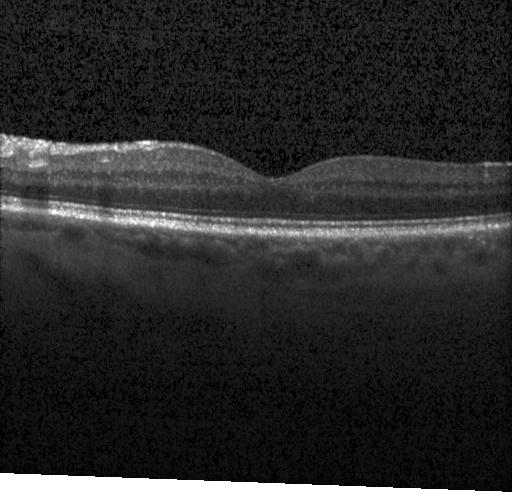
Finding: neither choroidal neovascularization, diabetic macular edema, nor drusen.